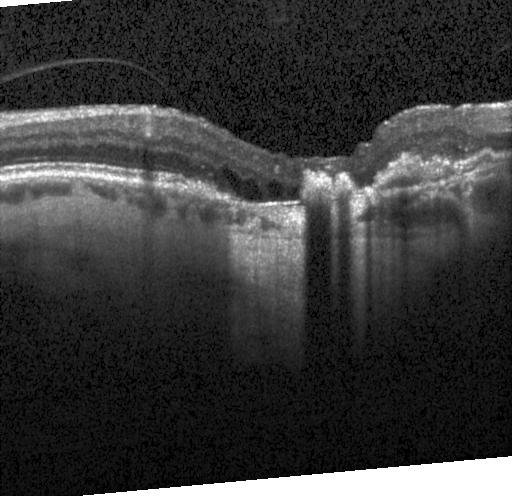
SD-OCT · retinal OCT cross-section · fovea-centered — OCT finding: a choroidal neovascular membrane.